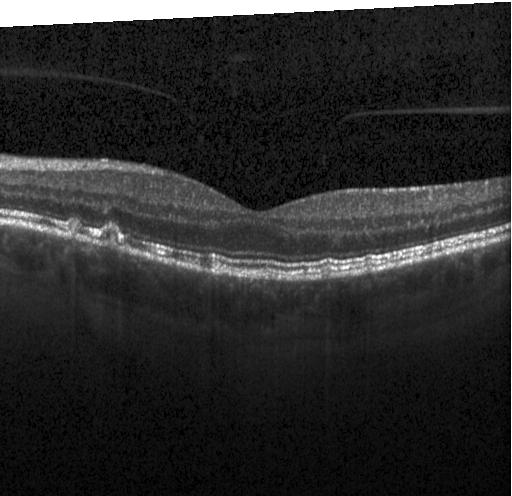 Heidelberg Spectralis, centered on the fovea, optical coherence tomography B-scan, spectral-domain OCT — Drusen.